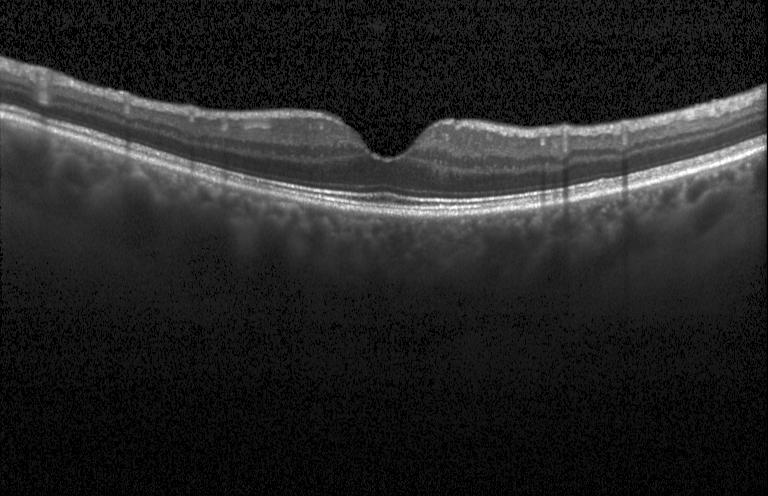

Heidelberg Spectralis OCT system; retinal OCT B-scan
Assessment: neither CNV, DME, nor drusen.